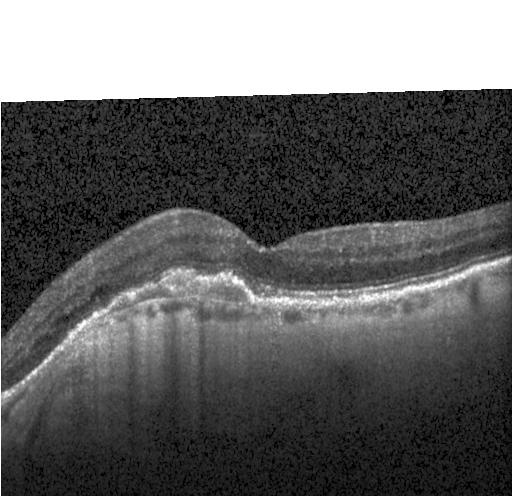

Fovea-centered · OCT line scan · SD-OCT · acquired on a Heidelberg Spectralis. Diagnosis: a choroidal neovascular membrane.